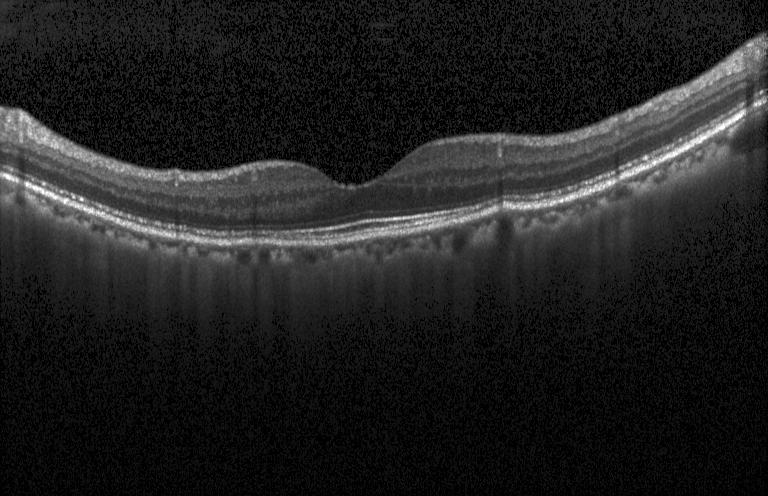

Horizontal scan through the fovea; Heidelberg Spectralis; optical coherence tomography scan; spectral-domain OCT. Assessment: no choroidal neovascularization, no diabetic macular edema, and no drusen.